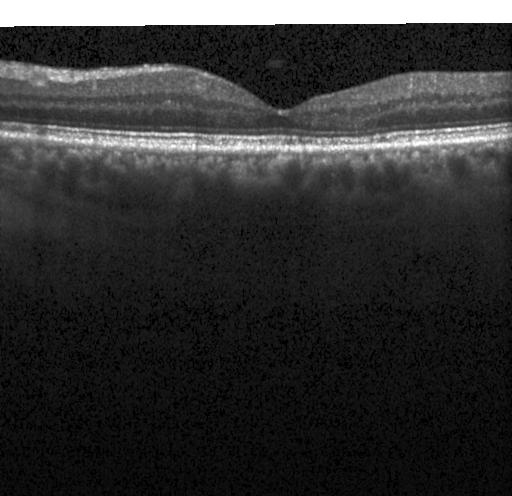
Retinal OCT cross-section
Diagnosis: no evidence of choroidal neovascularization, diabetic macular edema, or drusen.